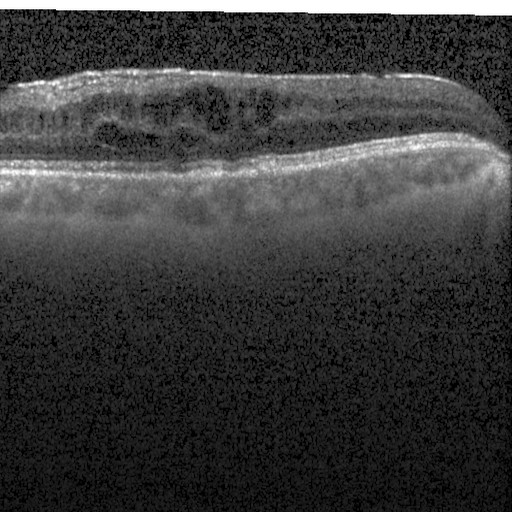

Macular OCT: diabetic macular edema.